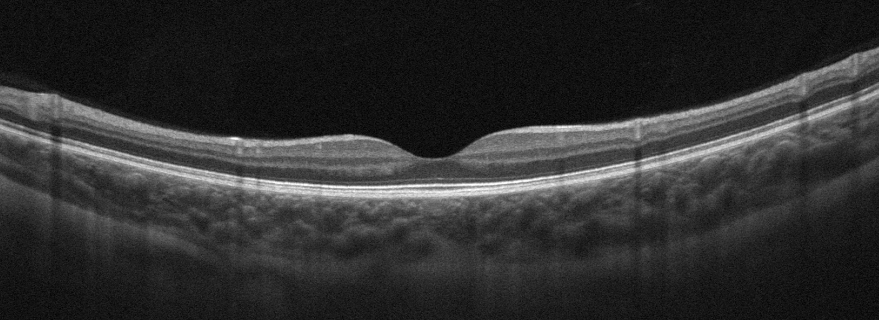
Assessment: absence of AMD, DME, ERM, RAO, RVO, and vitreomacular interface disease.